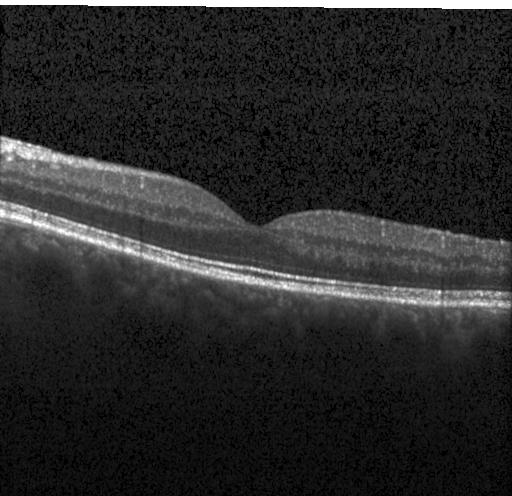
Finding: neither choroidal neovascularization, diabetic macular edema, nor drusen.